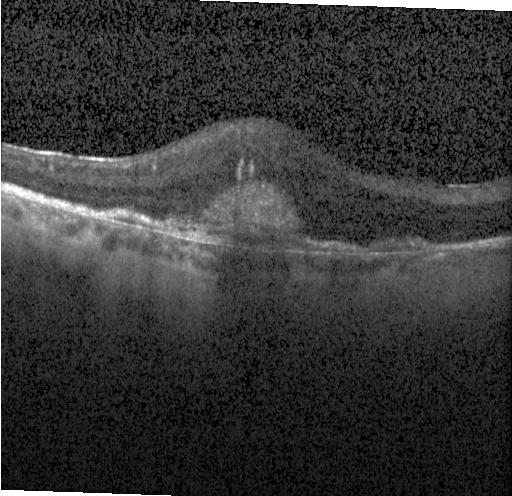

Retinal OCT B-scan, spectral-domain optical coherence tomography. Dx: a choroidal neovascular membrane.